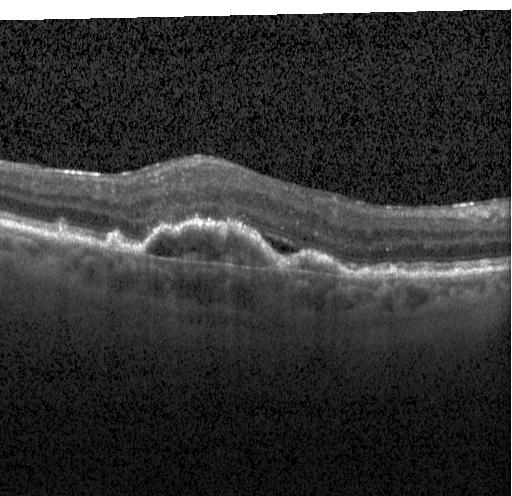
This B-scan demonstrates a choroidal neovascular membrane.